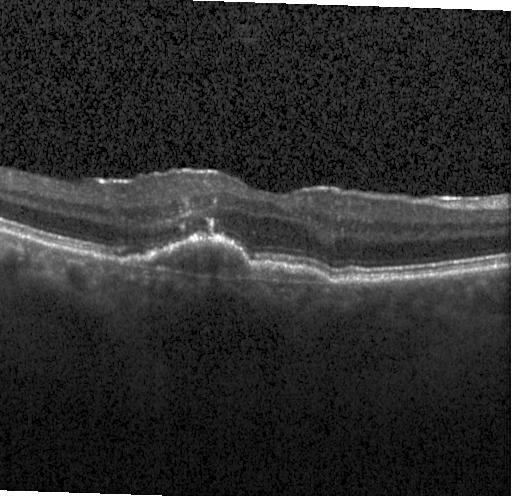

Retinal OCT B-scan. This B-scan demonstrates a choroidal neovascular membrane.